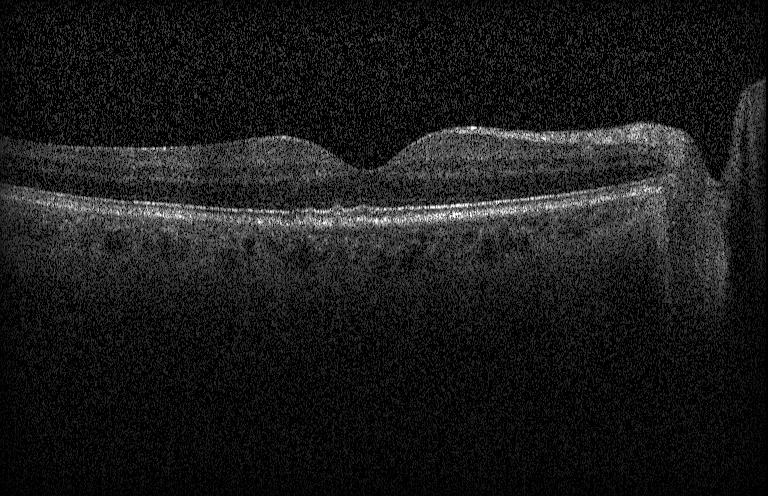 Heidelberg Spectralis OCT system; SD-OCT; through the macula; OCT B-scan. Finding: drusen.